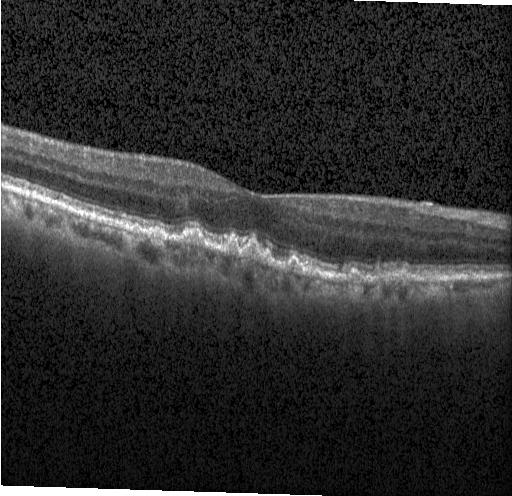

Macular OCT: sub-RPE drusenoid deposits.